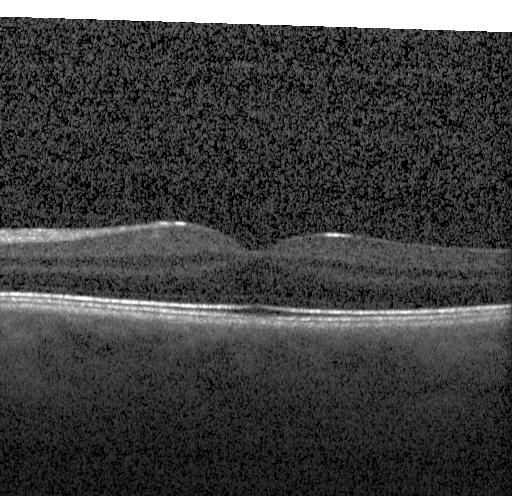
Retinal OCT cross-section · instrument: Heidelberg Spectralis · horizontal scan through the fovea · spectral-domain optical coherence tomography.
The scan shows neither CNV, DME, nor drusen.